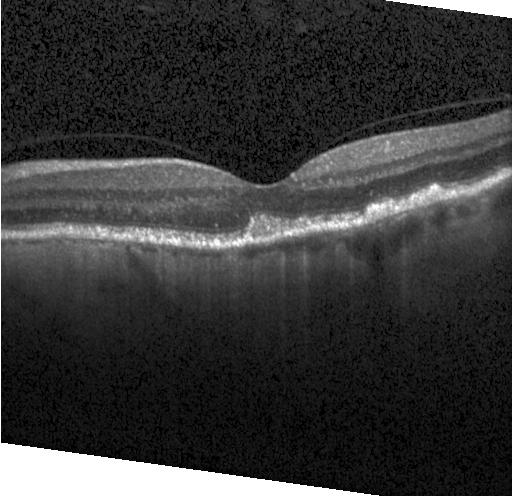

Retinal OCT cross-section showing sub-RPE drusenoid deposits.